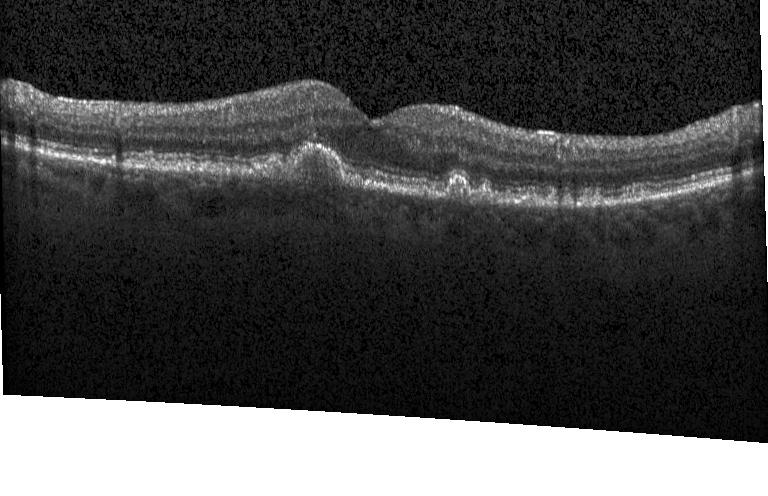

Finding: drusen.